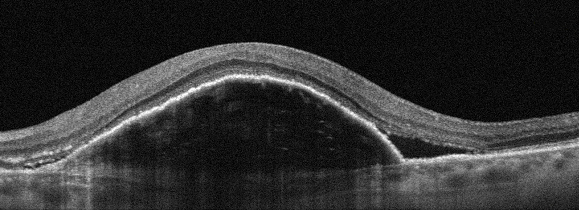

Oculus sinister; retinal OCT B-scan — Impression: age-related macular degeneration.